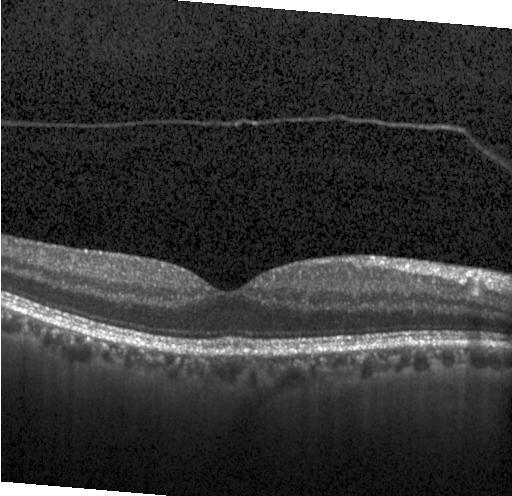 Finding: no evidence of choroidal neovascularization, diabetic macular edema, or drusen.